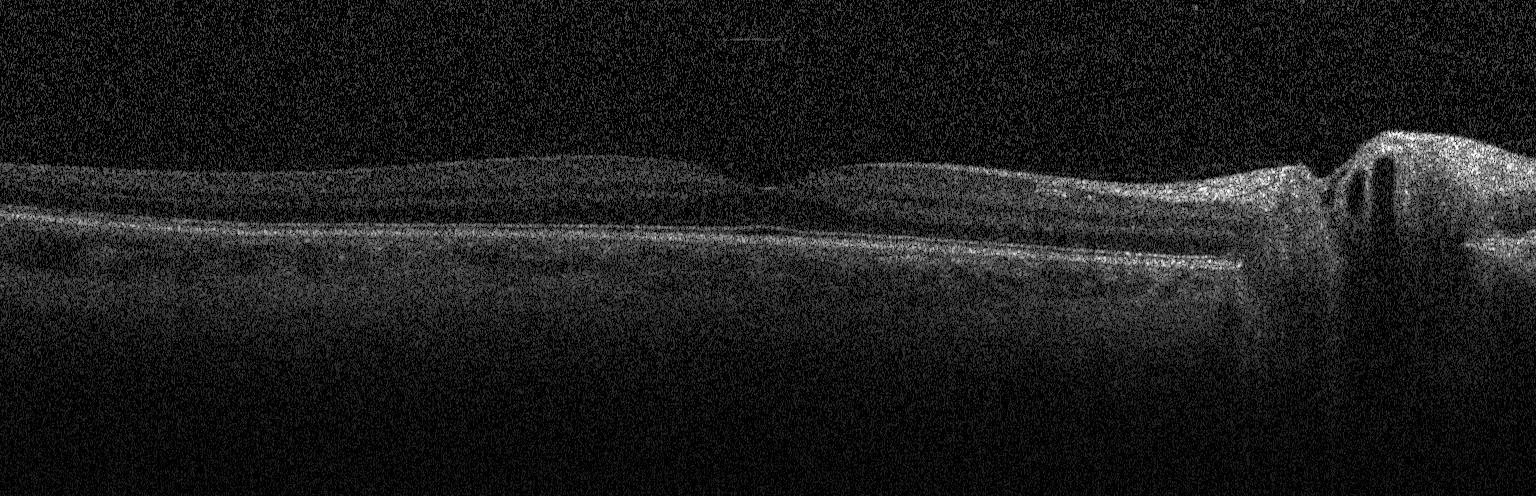

Macular scan; Heidelberg Spectralis OCT system; optical coherence tomography B-scan
No CNV, no DME, and no drusen.